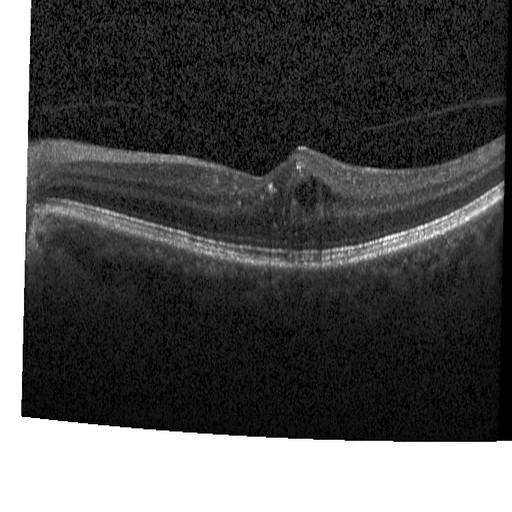

OCT B-scan
Finding: diabetic macular edema.